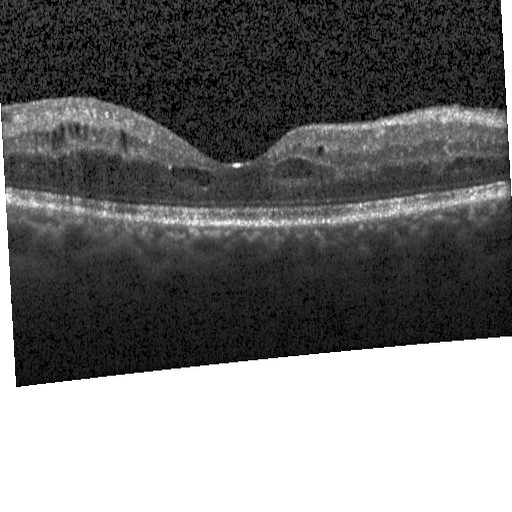 Diagnosis: diabetic macular edema.